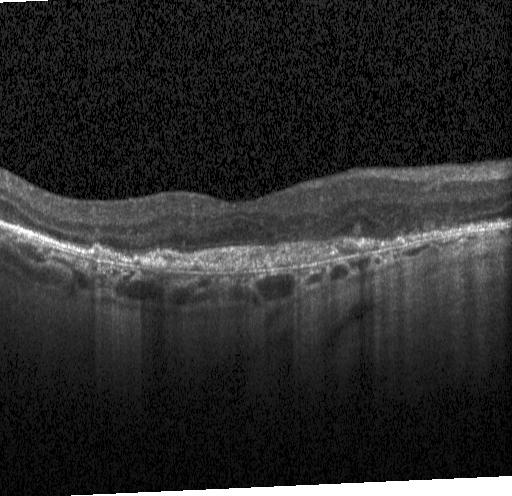 OCT finding: a choroidal neovascular membrane.